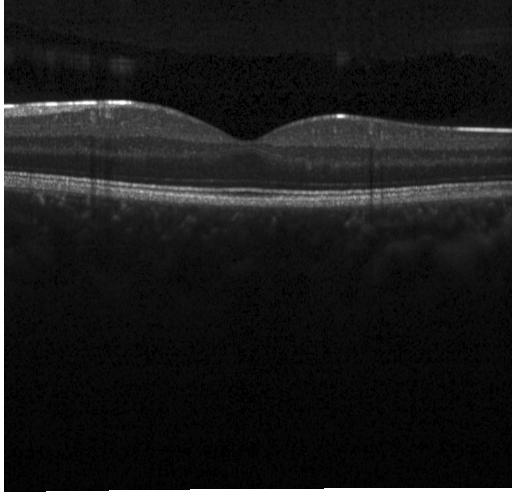
Optical coherence tomography B-scan · SD-OCT · Heidelberg Spectralis · fovea-centered — No CNV, no DME, and no drusen.